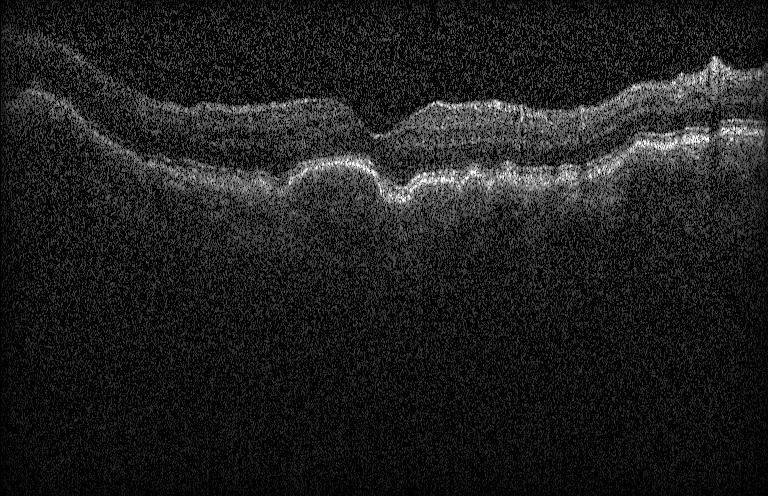

Retinal OCT cross-section showing sub-RPE drusenoid deposits.